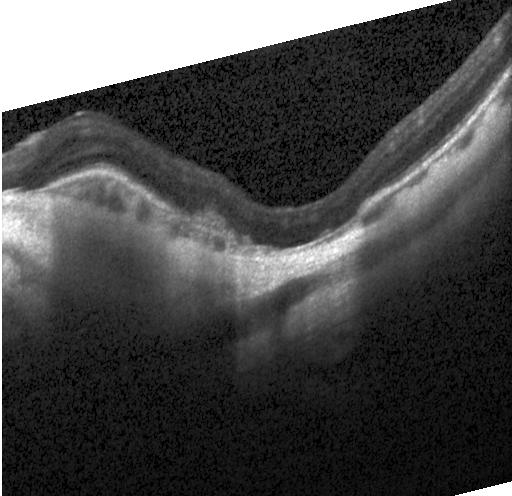
OCT B-scan.
Macular OCT: CNV.